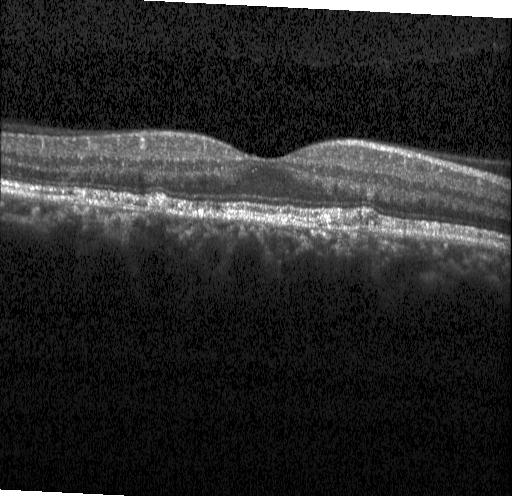

Optical coherence tomography scan — Assessment: drusen.